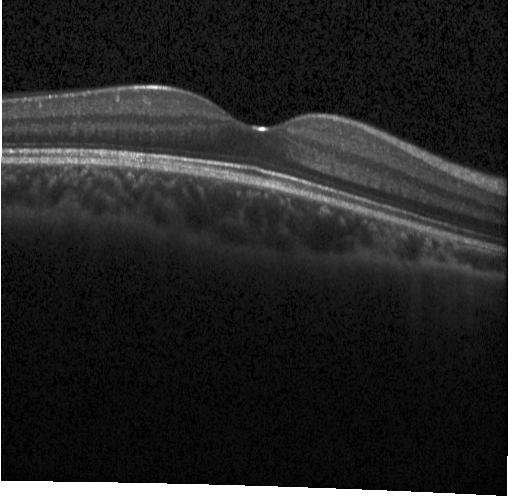

SD-OCT, macular scan, optical coherence tomography scan. OCT finding: no CNV, no DME, and no drusen.